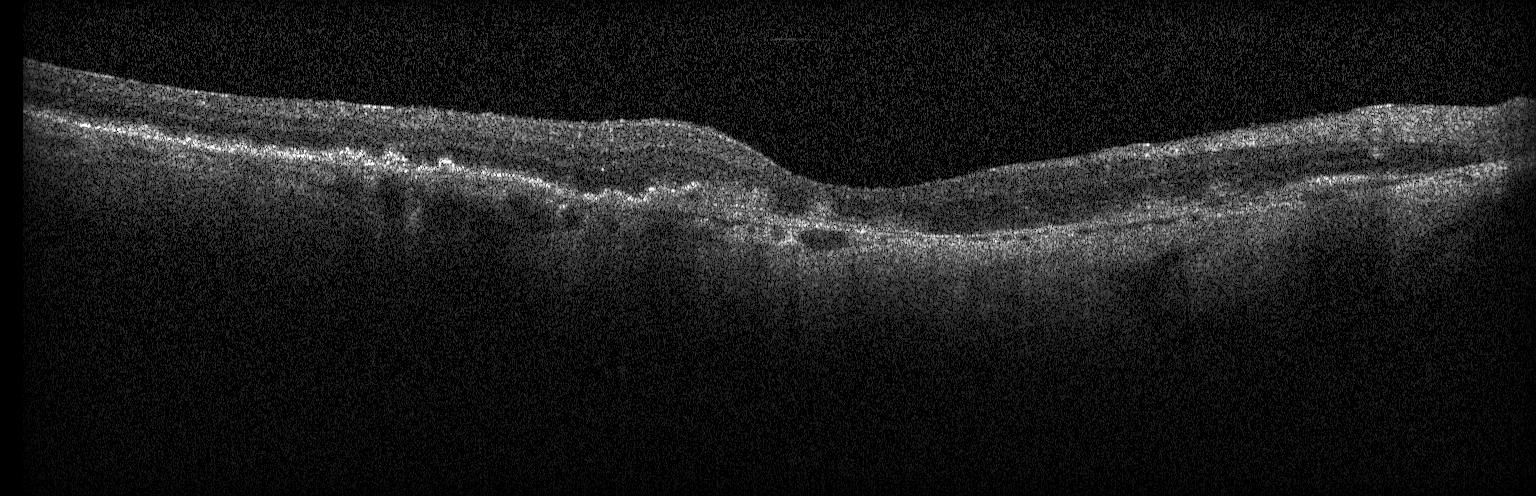 OCT line scan · spectral-domain OCT · macular scan · acquired on a Heidelberg Spectralis. Dx: a choroidal neovascular membrane.